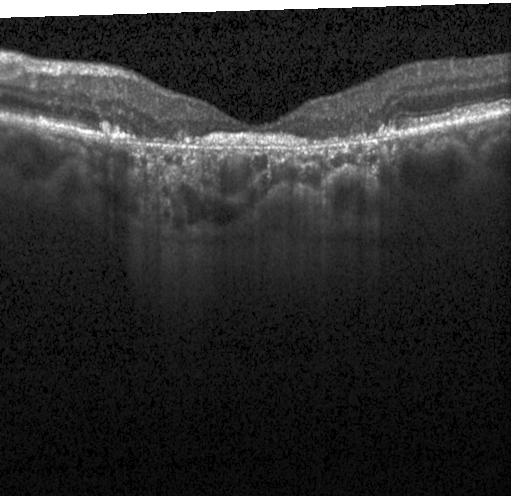

Diagnosis: CNV.